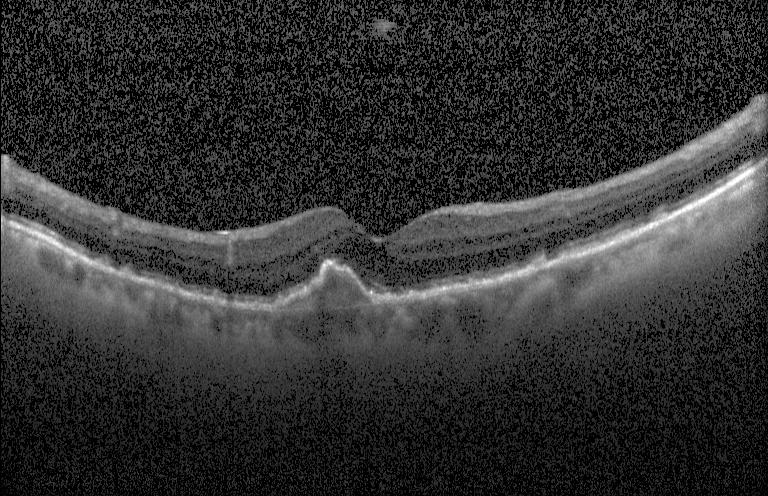

Assessment: choroidal neovascularization.